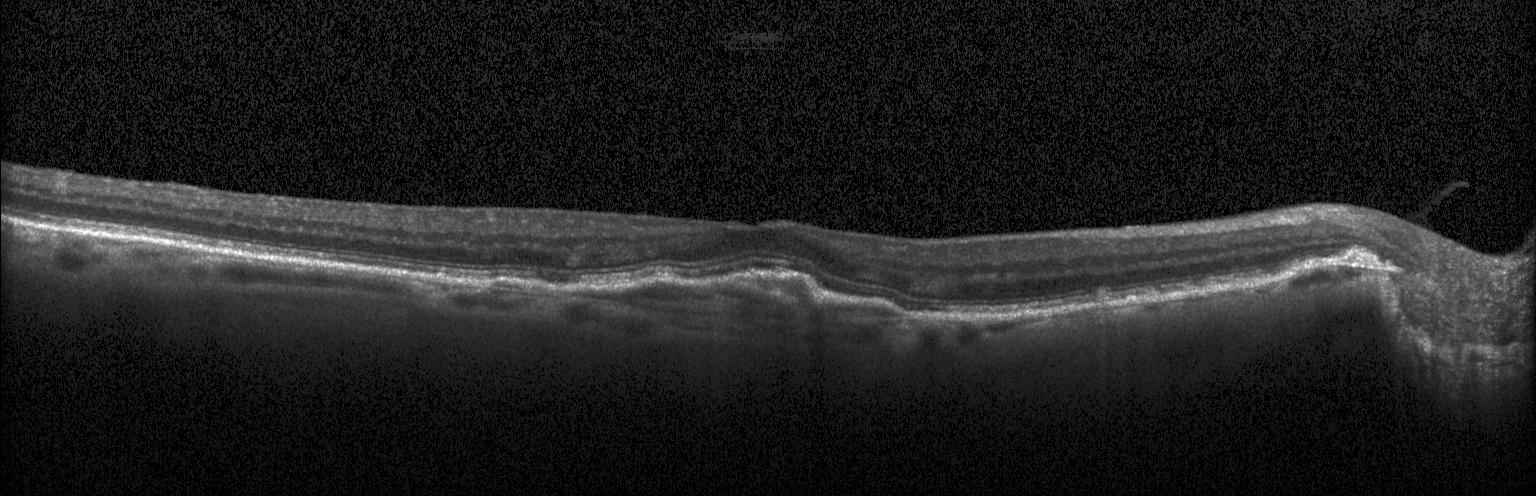 Instrument: Heidelberg Spectralis, optical coherence tomography scan, macular scan. Finding: a choroidal neovascular membrane.